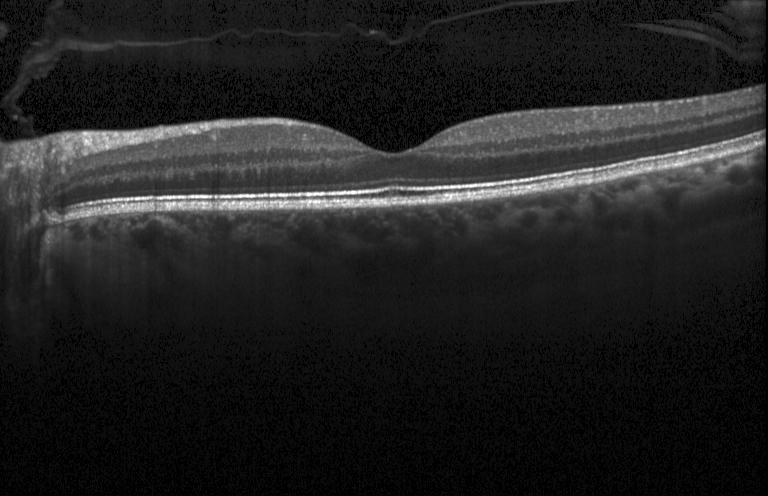
Optical coherence tomography B-scan; spectral-domain OCT
Finding: no evidence of choroidal neovascularization, diabetic macular edema, or drusen.